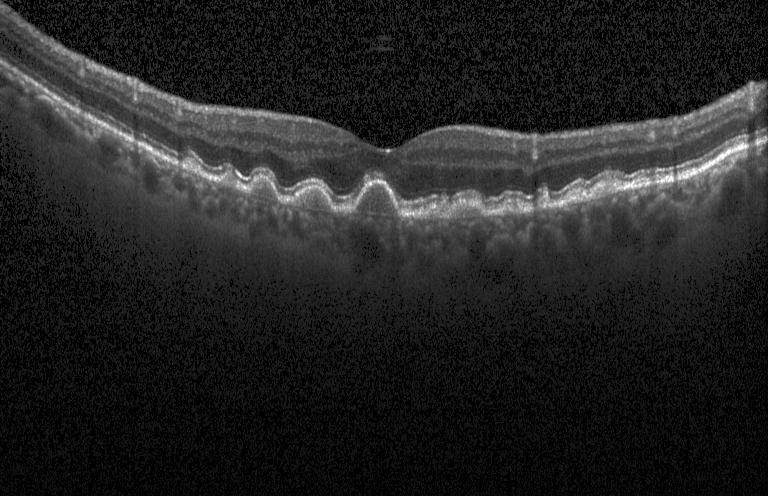 Horizontal scan through the fovea. Retinal OCT cross-section — Dx: sub-RPE drusenoid deposits.